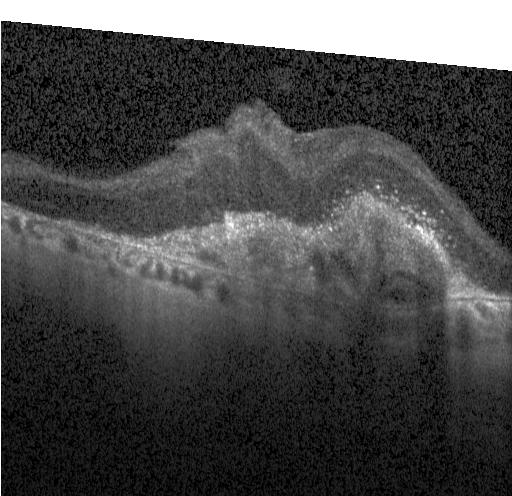 Heidelberg Spectralis; OCT line scan — A choroidal neovascular membrane.